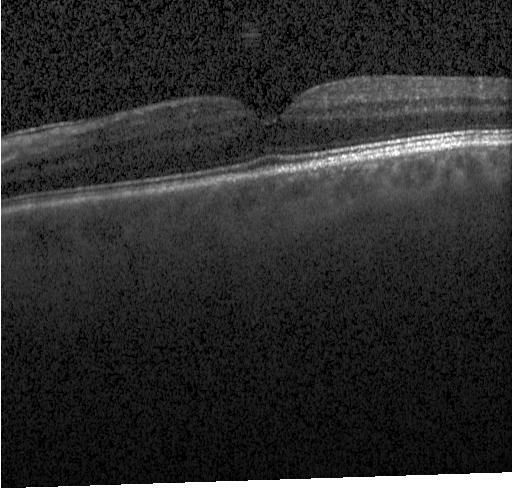 Impression: no CNV, DME, or drusen.